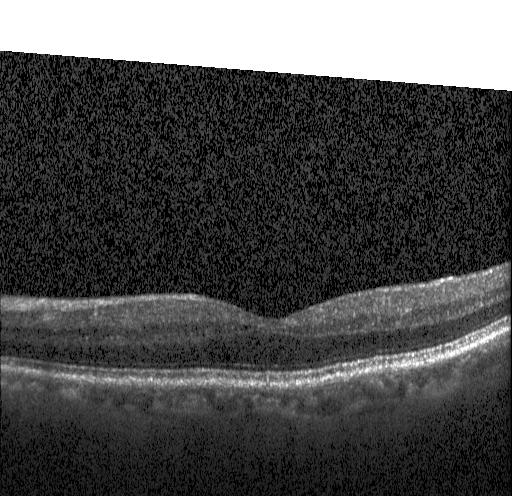
Spectral-domain OCT B-scan: neither choroidal neovascularization, diabetic macular edema, nor drusen.